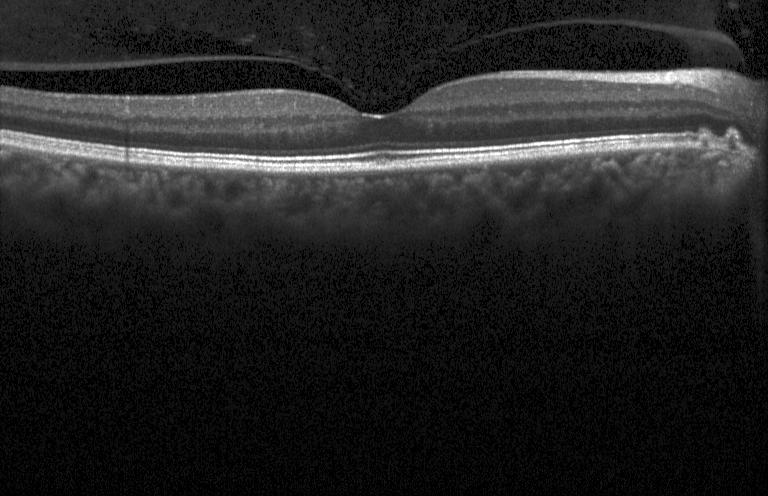 Acquired on a Heidelberg Spectralis; retinal OCT B-scan — OCT finding: no choroidal neovascularization, no diabetic macular edema, and no drusen.